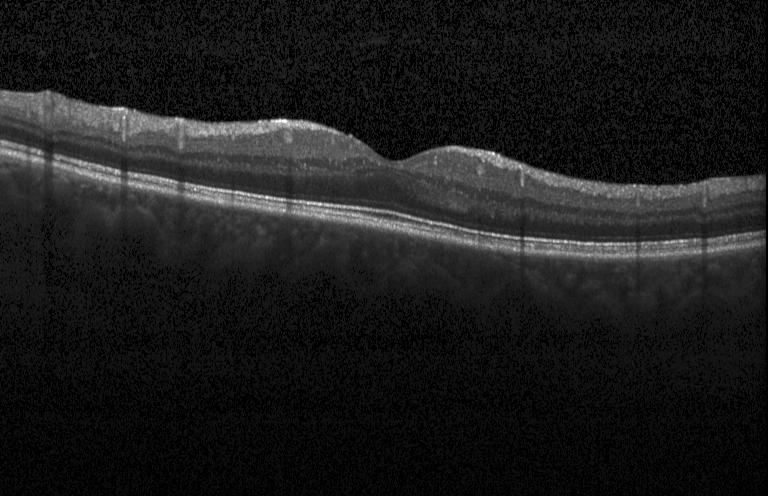 The scan shows no choroidal neovascularization, diabetic macular edema, or drusen.